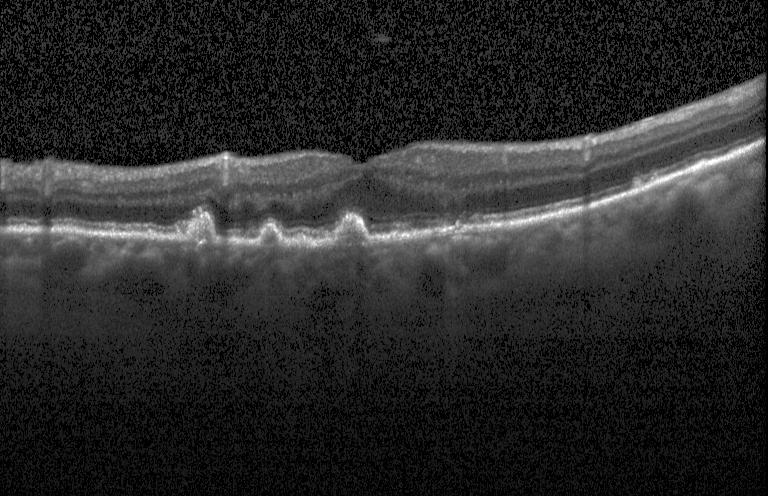 OCT B-scan
Dx: multiple drusen.